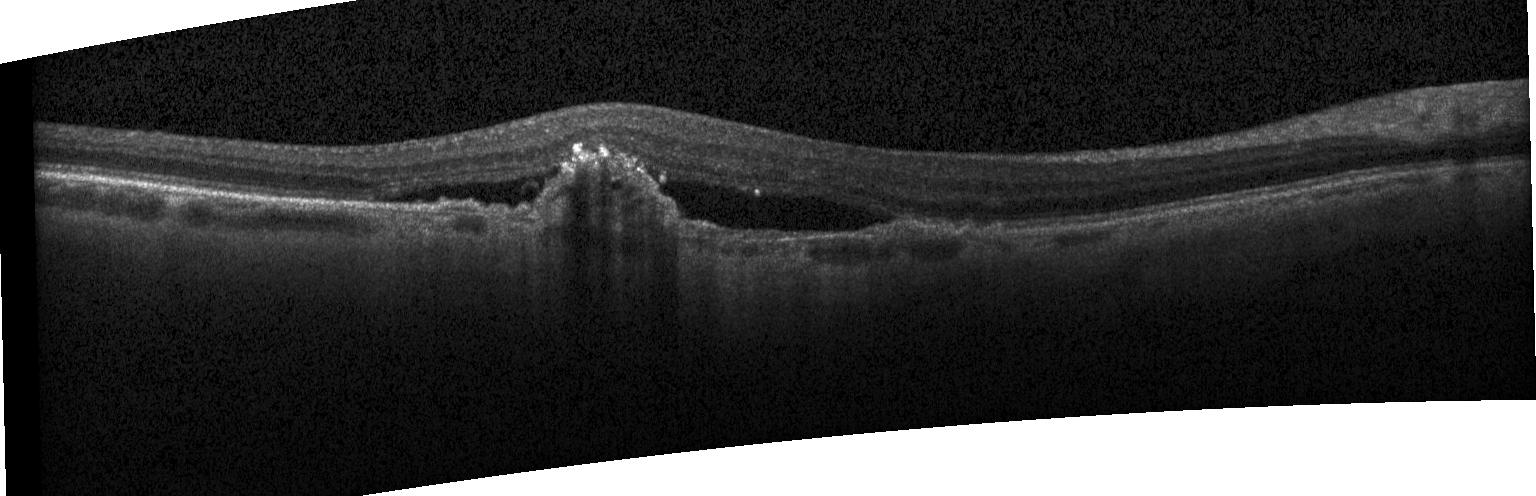

OCT B-scan · SD-OCT
OCT finding: CNV.